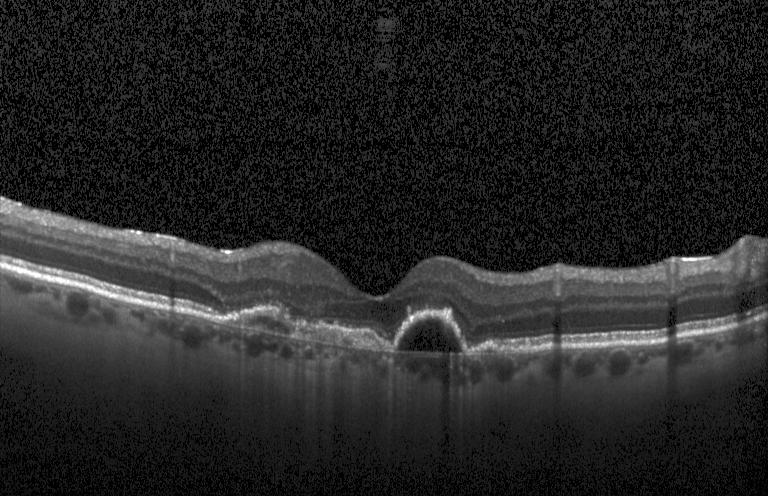 Dx: a choroidal neovascular membrane.